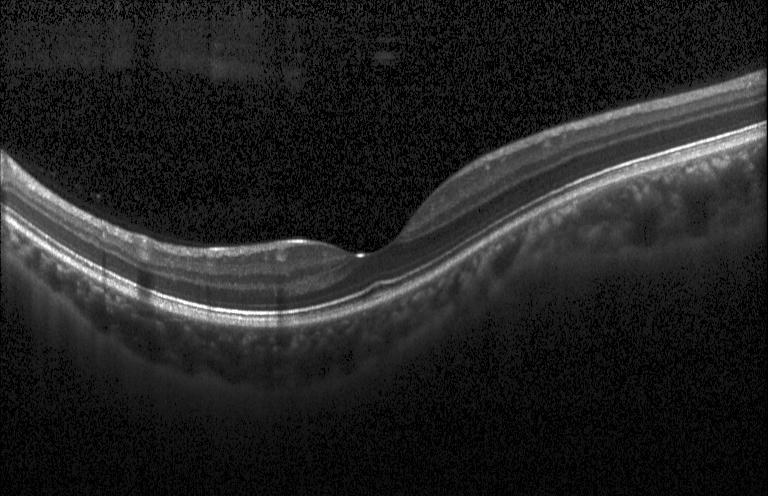
OCT line scan. This B-scan demonstrates no choroidal neovascularization, diabetic macular edema, or drusen.